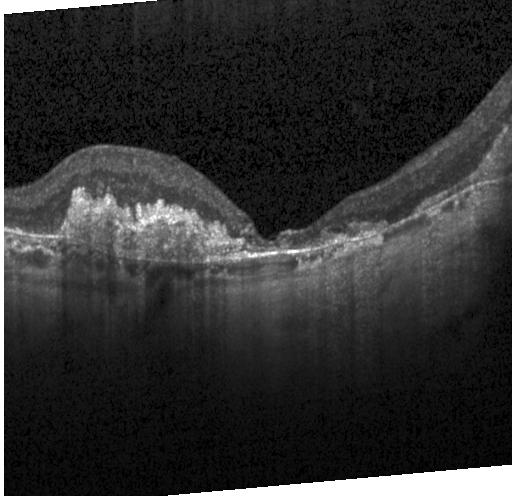 OCT B-scan — Macular OCT: CNV.